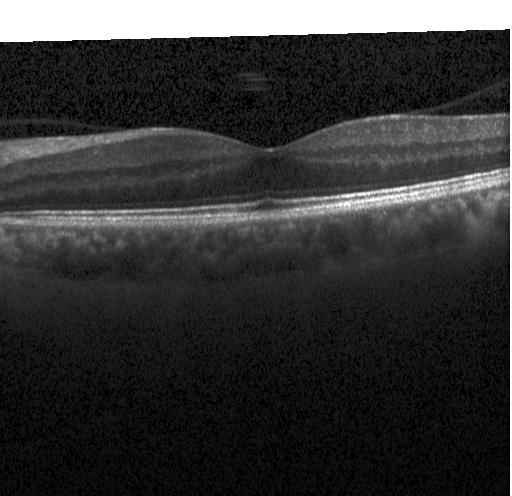 SD-OCT; centered on the fovea; retinal OCT B-scan. Dx: no choroidal neovascularization, diabetic macular edema, or drusen.